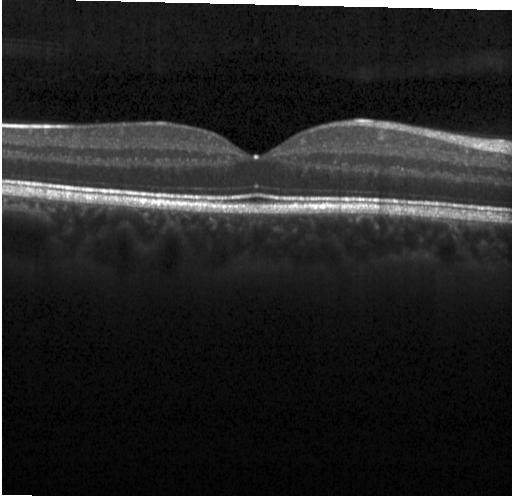 Heidelberg Spectralis OCT system · macular scan · retinal OCT B-scan · spectral-domain OCT — Dx: no evidence of CNV, DME, or drusen.